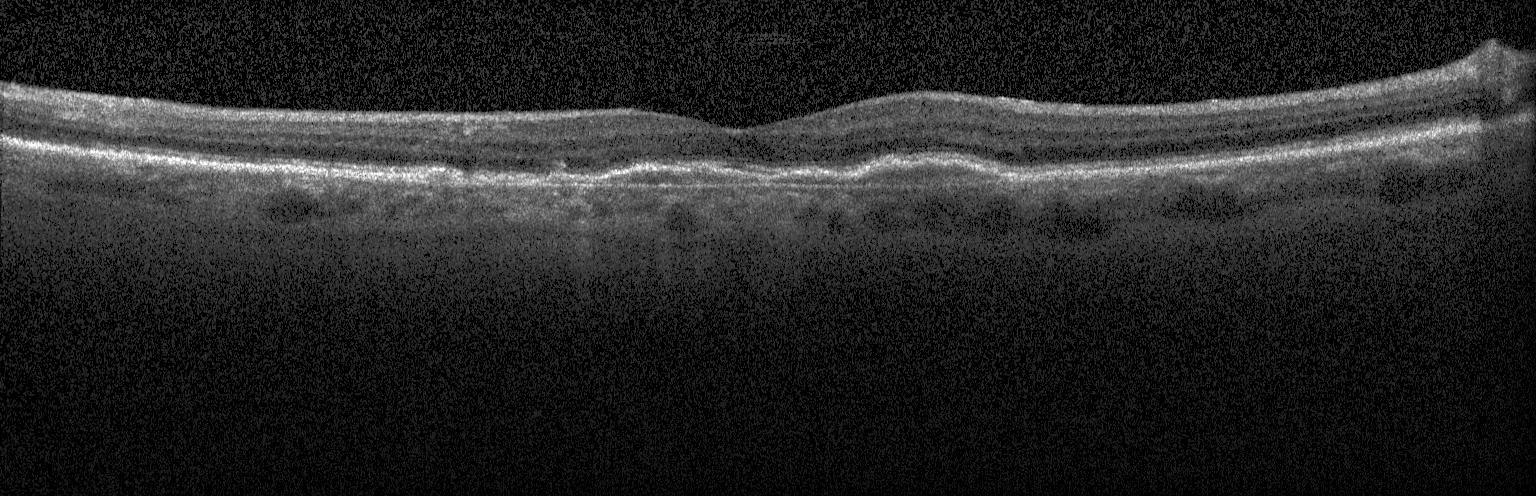 OCT B-scan; spectral-domain OCT; Heidelberg Spectralis OCT system.
This B-scan demonstrates a choroidal neovascular membrane.